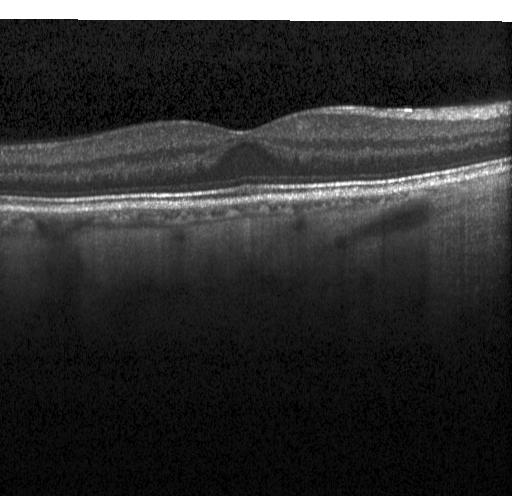
SD-OCT. Optical coherence tomography B-scan — Impression: no CNV, DME, or drusen.